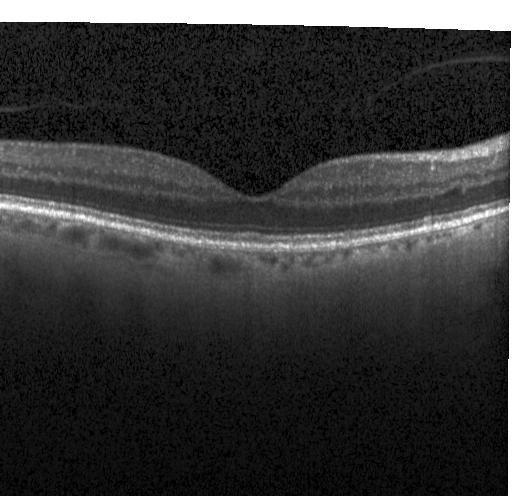

Acquired on a Heidelberg Spectralis, fovea-centered, SD-OCT, optical coherence tomography scan — Macular OCT: no choroidal neovascularization, diabetic macular edema, or drusen.